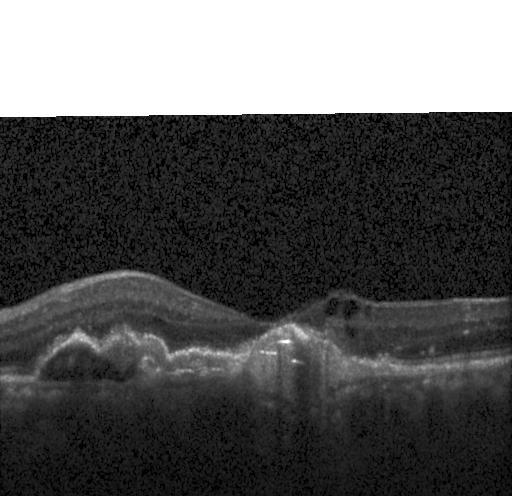
Optical coherence tomography B-scan; macular scan — Assessment: a choroidal neovascular membrane.